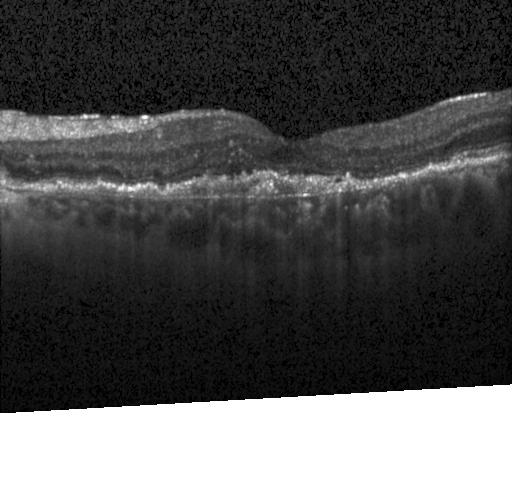 The scan shows CNV.